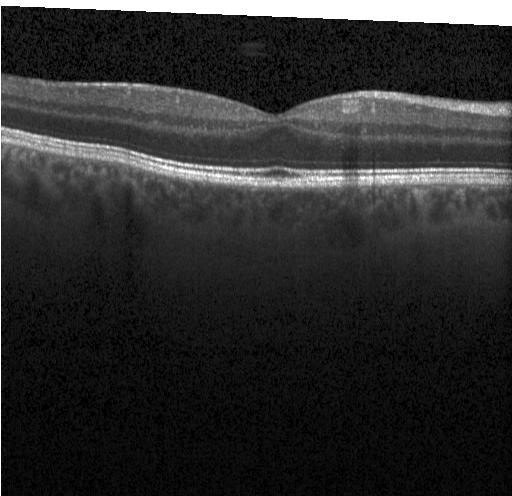

OCT B-scan. Assessment: no choroidal neovascularization, no diabetic macular edema, and no drusen.